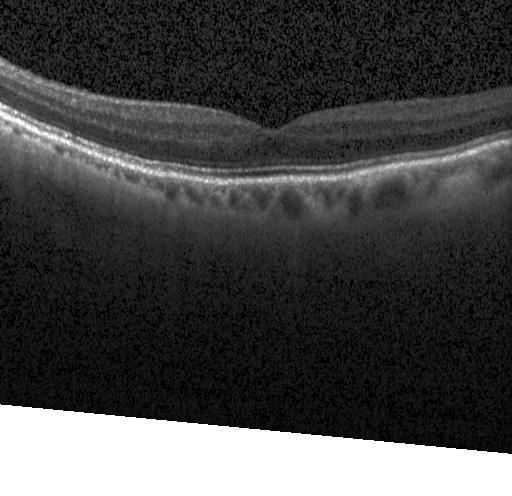
Retinal OCT B-scan.
The scan shows no choroidal neovascularization, diabetic macular edema, or drusen.